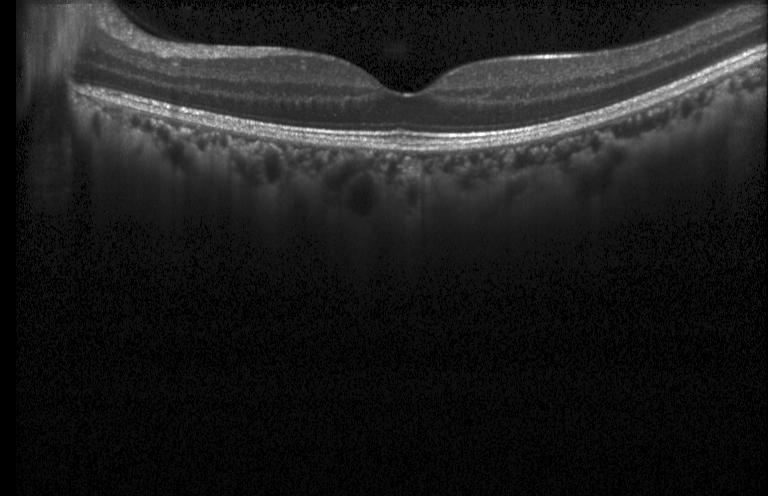
Neither CNV, DME, nor drusen.